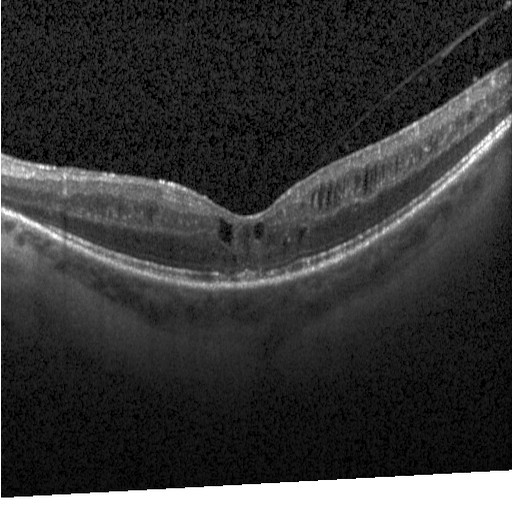
Heidelberg Spectralis OCT system · retinal OCT cross-section · spectral-domain OCT · centered on the fovea. Finding: diabetic macular edema (DME).